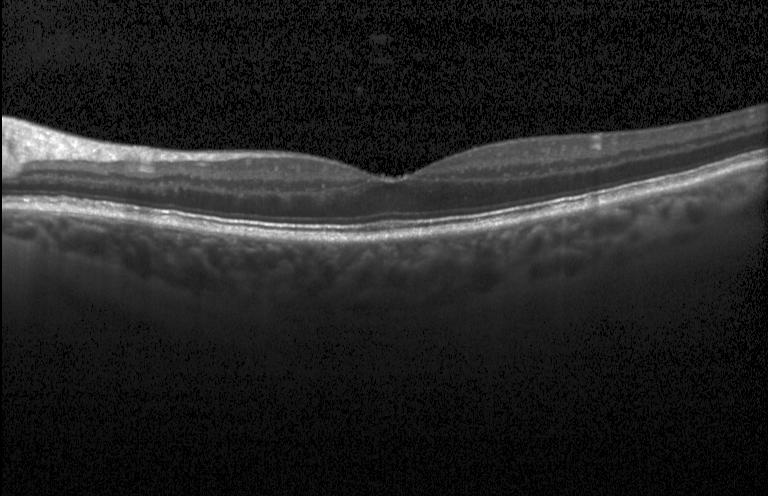
Finding: neither choroidal neovascularization, diabetic macular edema, nor drusen.